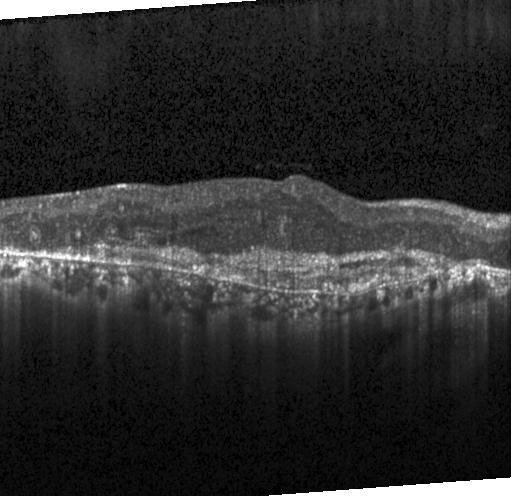 Retinal OCT cross-section. This B-scan demonstrates CNV.